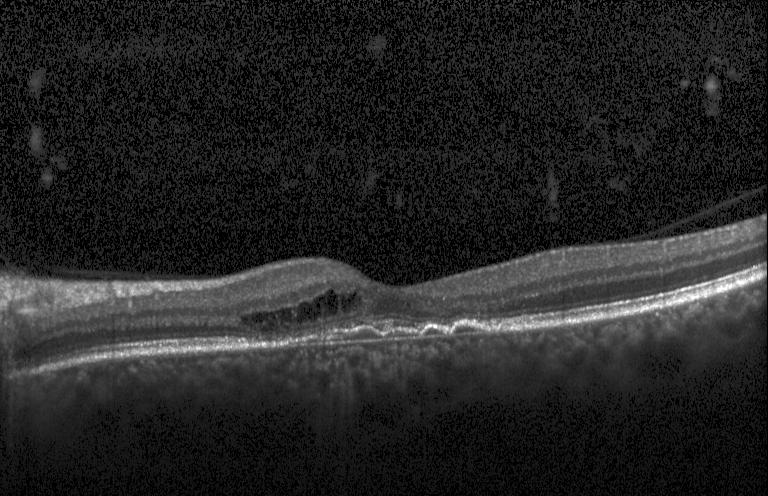 OCT B-scan
Impression: a choroidal neovascular membrane.